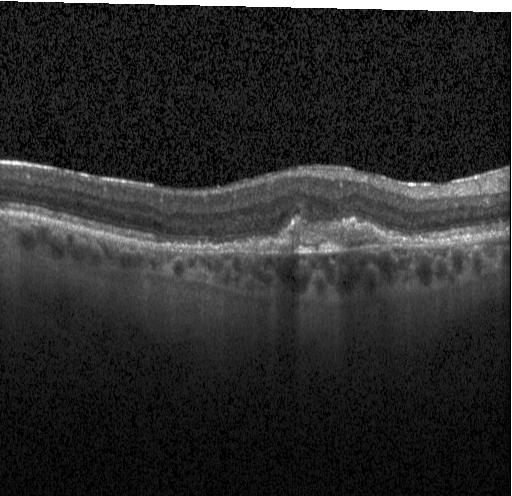

OCT line scan
Dx: choroidal neovascularization (CNV).